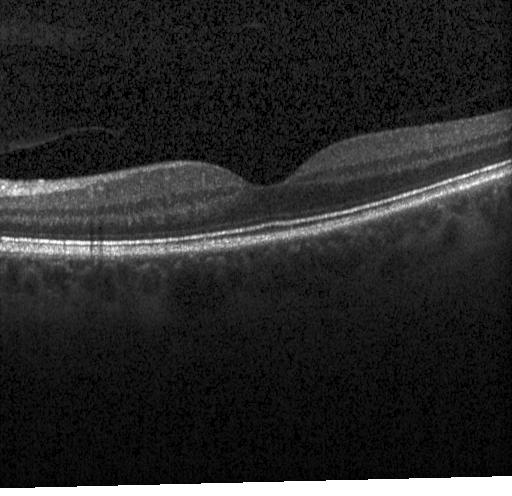
Optical coherence tomography scan — Finding: no evidence of choroidal neovascularization, diabetic macular edema, or drusen.